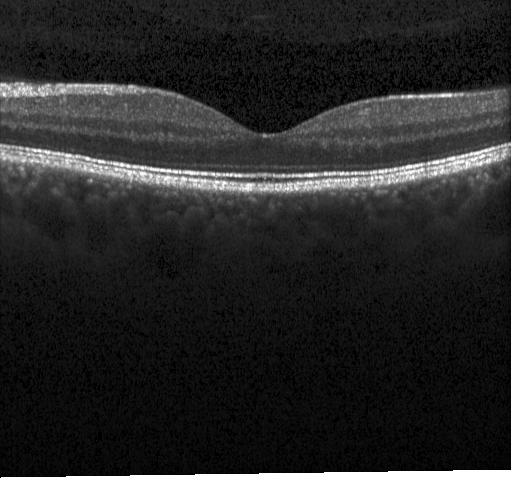 Heidelberg Spectralis, macular scan, retinal OCT B-scan. Impression: no evidence of choroidal neovascularization, diabetic macular edema, or drusen.